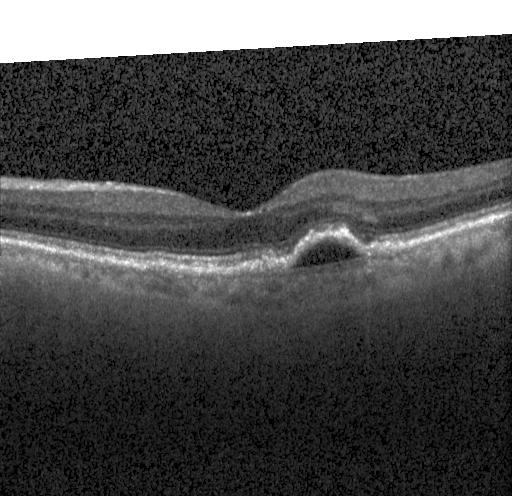

Macular scan; optical coherence tomography scan; SD-OCT; instrument: Heidelberg Spectralis. Finding: CNV.